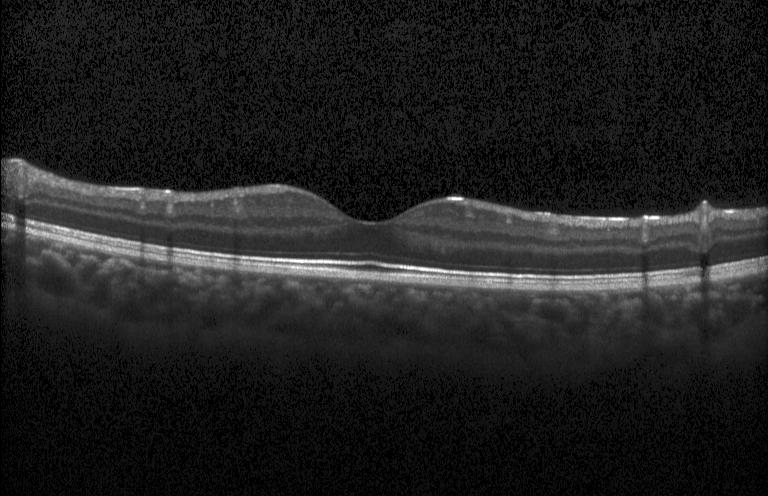
Retinal OCT cross-section
Impression: neither choroidal neovascularization, diabetic macular edema, nor drusen.